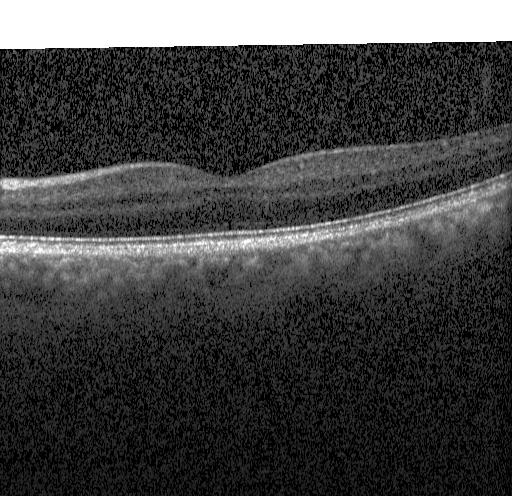
OCT line scan
This B-scan demonstrates no evidence of choroidal neovascularization, diabetic macular edema, or drusen.